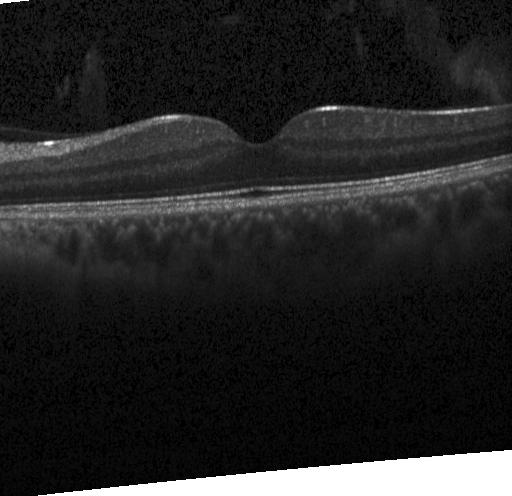
SD-OCT, fovea-centered, optical coherence tomography scan, Heidelberg Spectralis. No evidence of choroidal neovascularization, diabetic macular edema, or drusen.